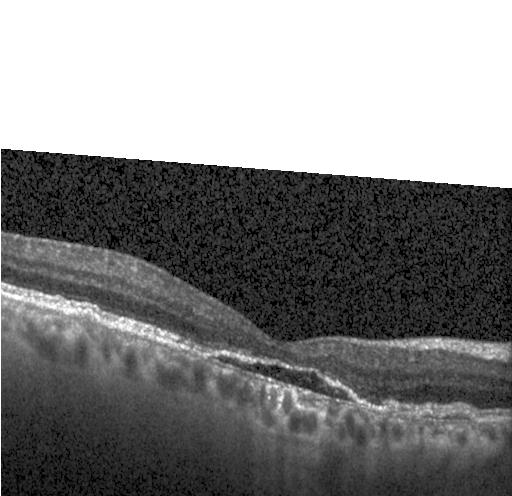

Retinal OCT cross-section. Heidelberg Spectralis OCT system.
Assessment: choroidal neovascularization.